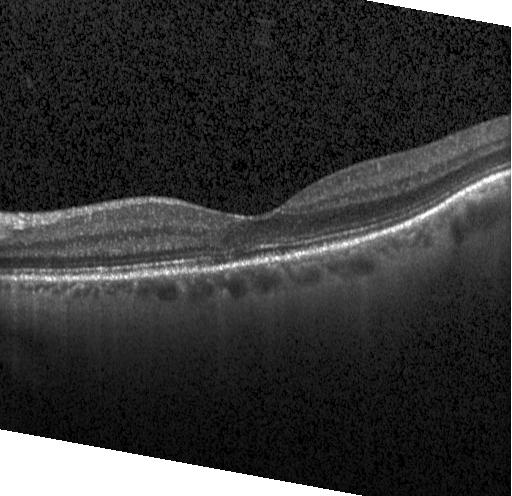
Retinal OCT cross-section showing no choroidal neovascularization, no diabetic macular edema, and no drusen.